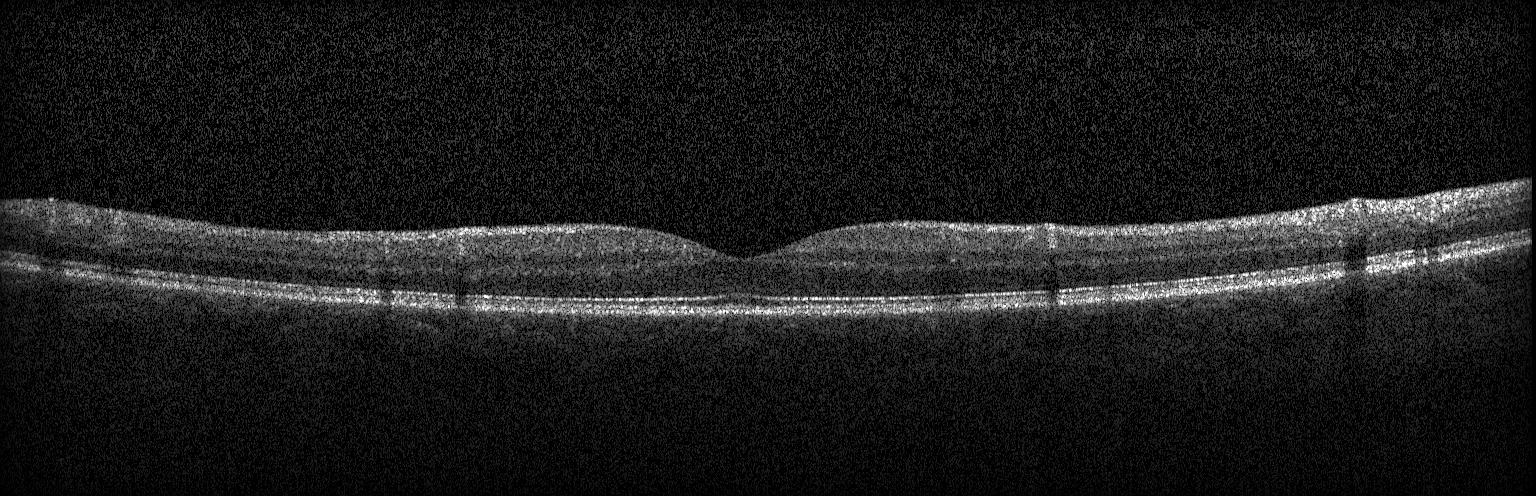
Diagnosis: no evidence of CNV, DME, or drusen.